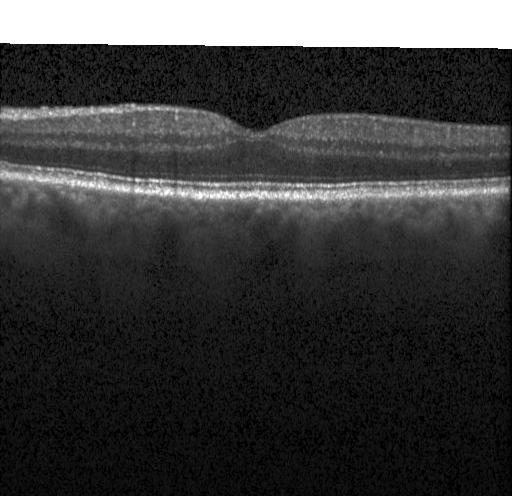
Optical coherence tomography B-scan · through the macula — Impression: no choroidal neovascularization, no diabetic macular edema, and no drusen.